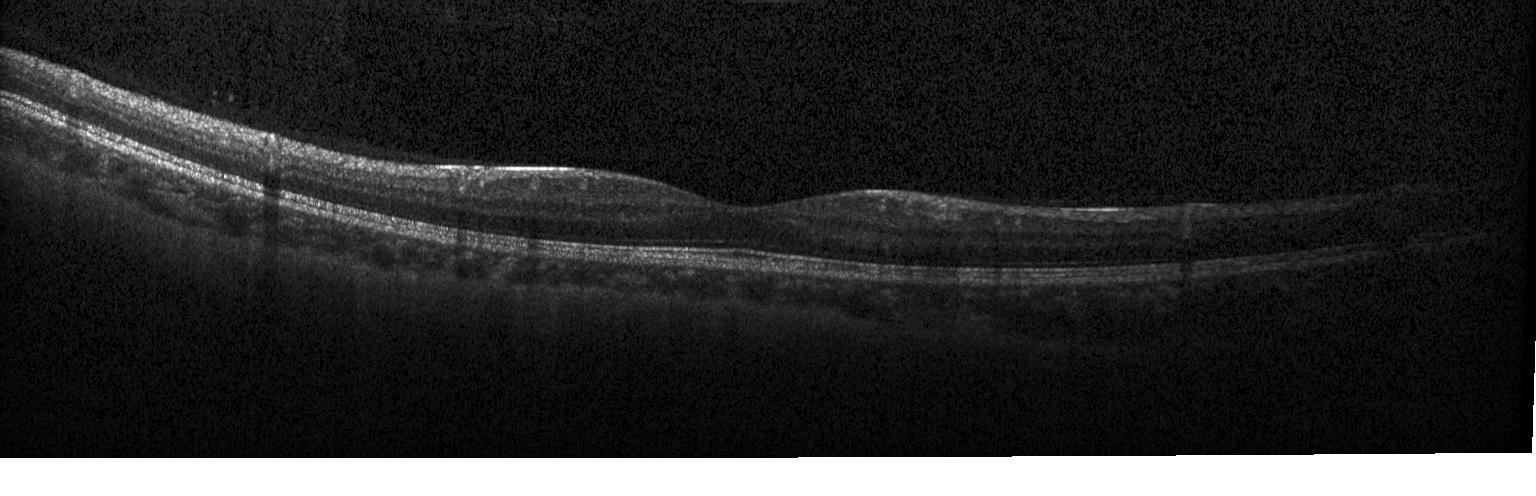

OCT B-scan — The scan shows no CNV, DME, or drusen.